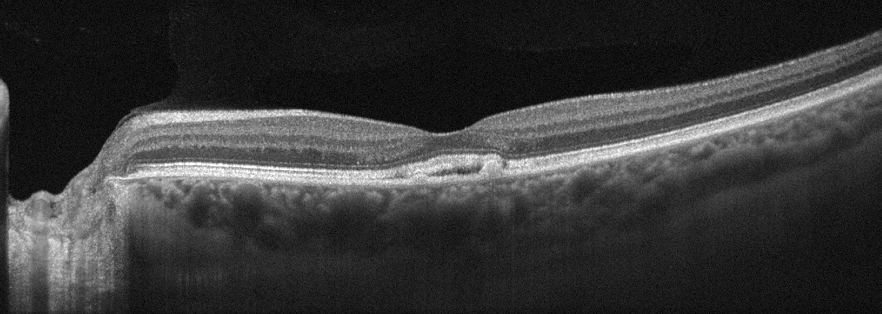 OCT line scan, OS
Diagnosis: age-related macular degeneration.